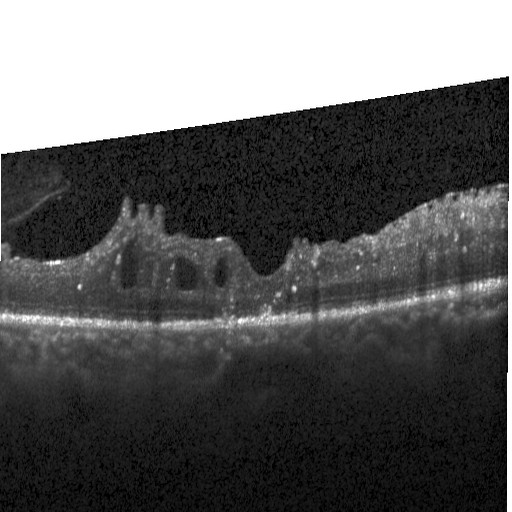 Retinal OCT B-scan, spectral-domain OCT — Finding: diabetic macular edema (DME).